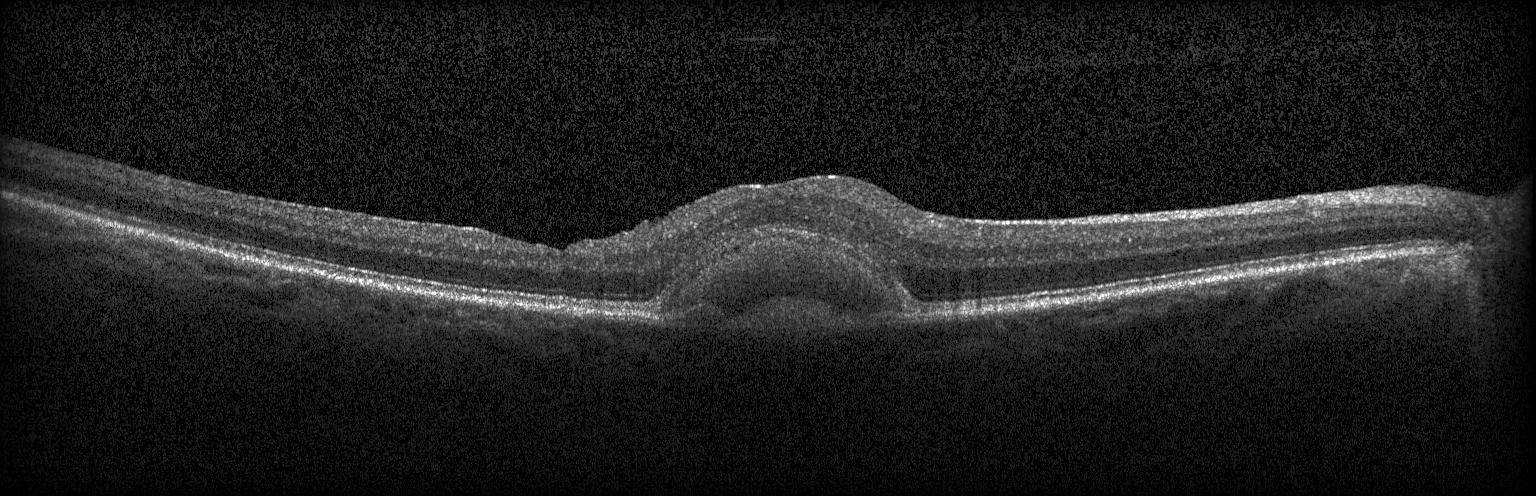

Retinal OCT cross-section · spectral-domain optical coherence tomography · macular scan.
Diagnosis: a choroidal neovascular membrane.